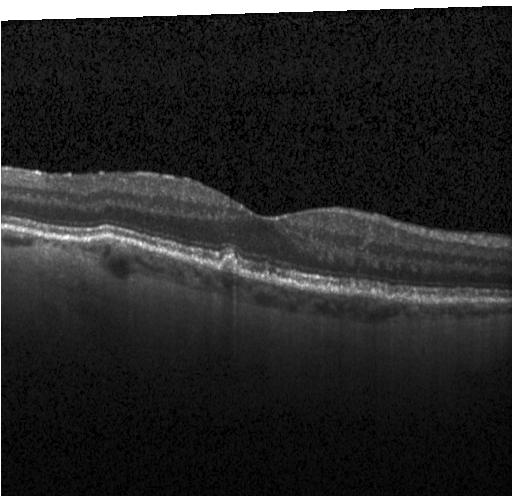
Retinal OCT cross-section showing multiple drusen.